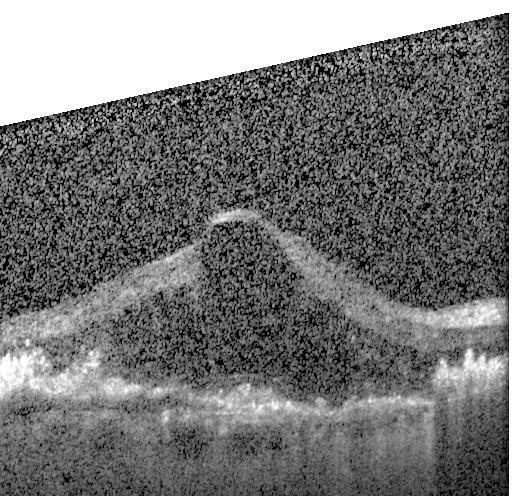
Assessment: CNV.